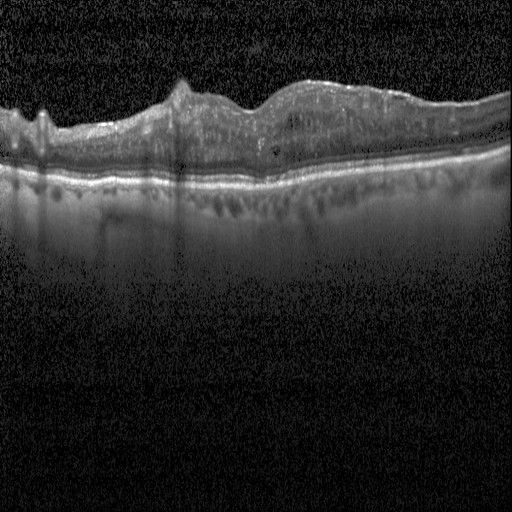

Instrument: Heidelberg Spectralis, through the macula, SD-OCT, OCT line scan
Finding: diabetic macular edema.